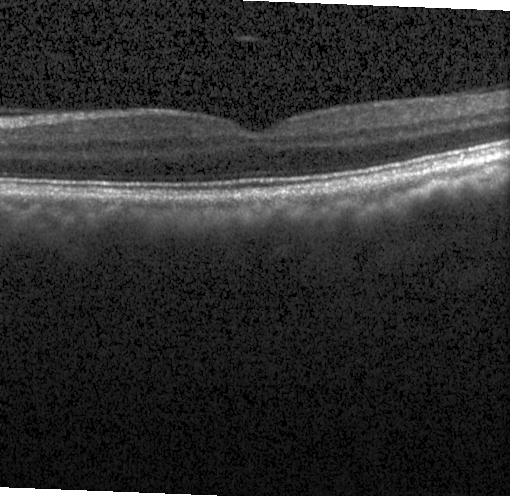

Optical coherence tomography B-scan. Finding: no CNV, no DME, and no drusen.